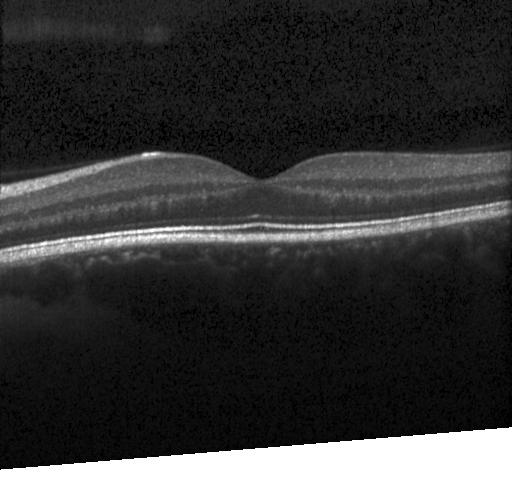 Impression: no evidence of choroidal neovascularization, diabetic macular edema, or drusen.